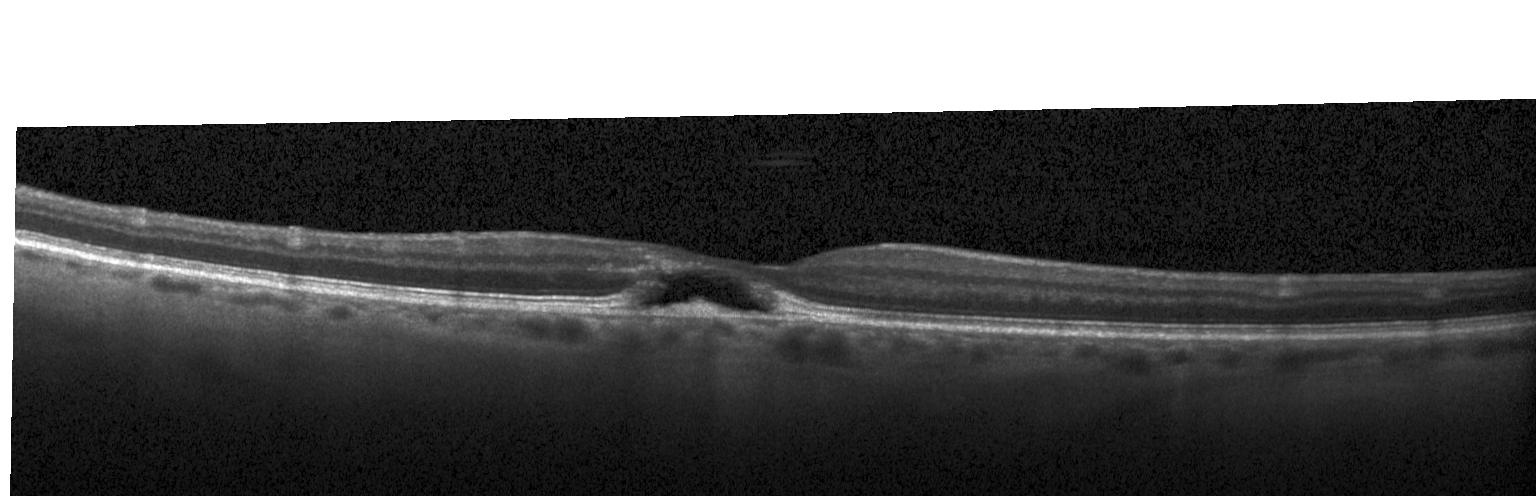
Spectral-domain OCT, optical coherence tomography B-scan. Diagnosis: a choroidal neovascular membrane.